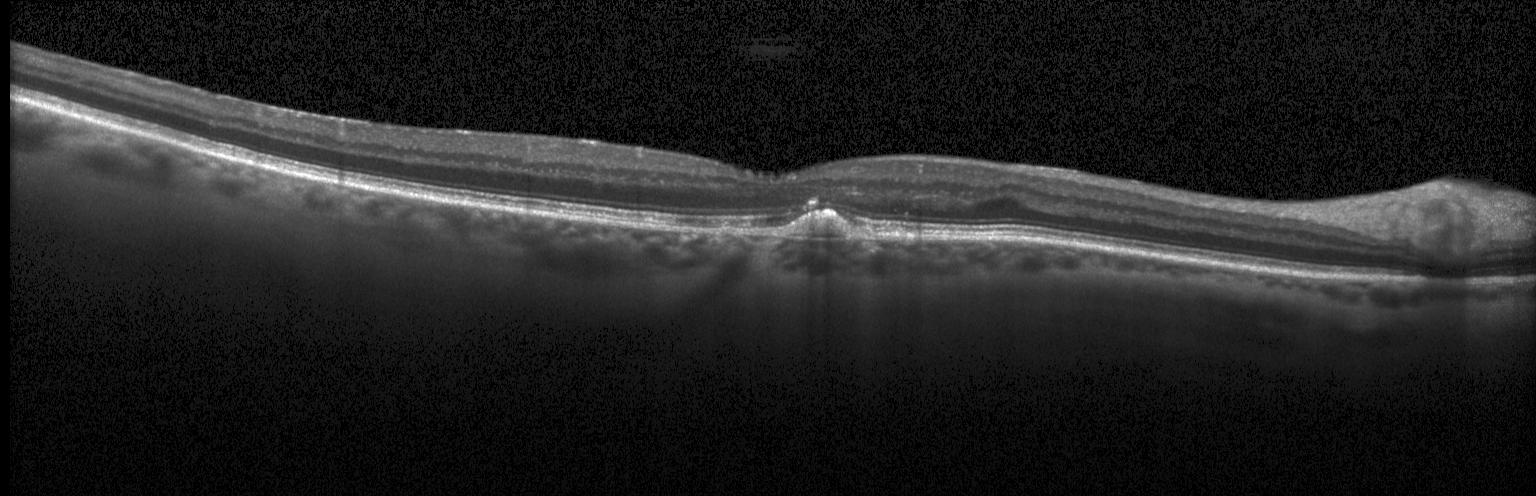 Instrument: Heidelberg Spectralis, SD-OCT, retinal OCT B-scan, horizontal scan through the fovea.
Finding: a choroidal neovascular membrane.